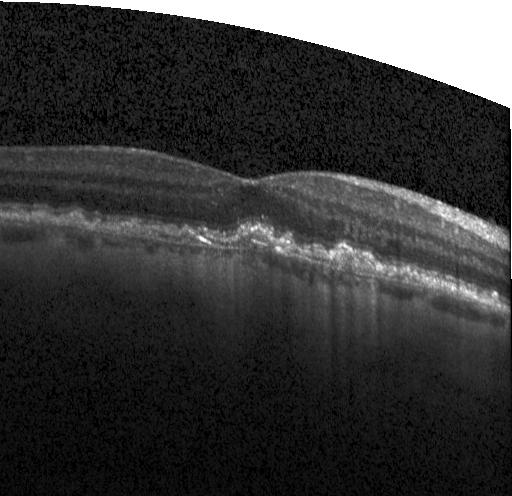

Centered on the fovea · OCT B-scan · acquired on a Heidelberg Spectralis.
This B-scan demonstrates a choroidal neovascular membrane.